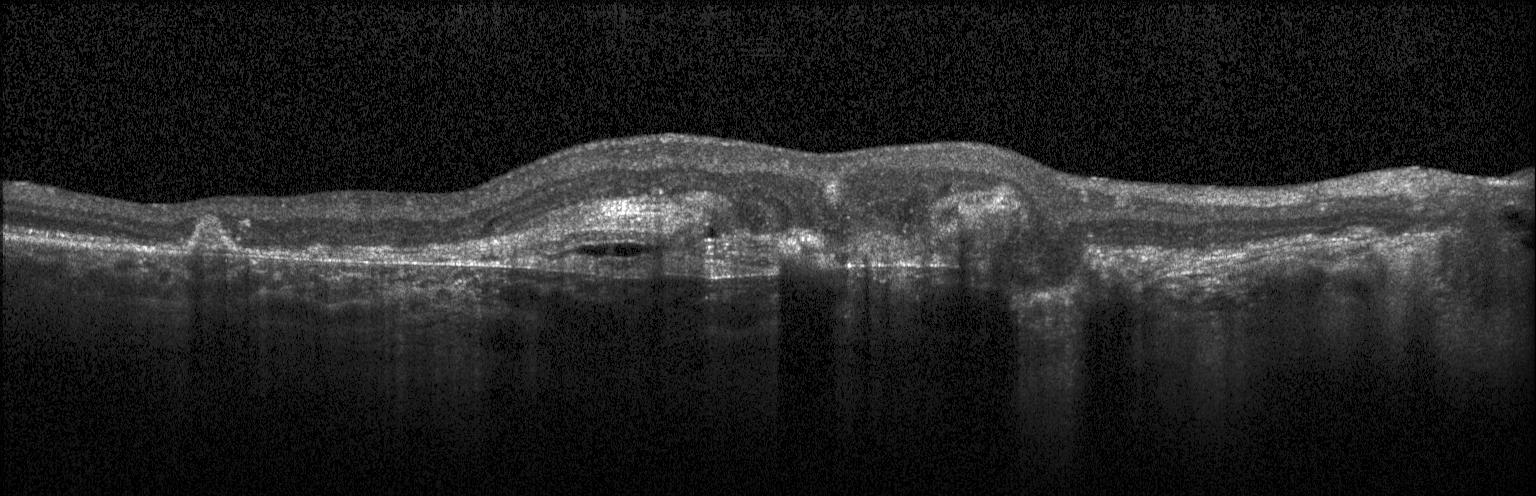

Horizontal scan through the fovea, Heidelberg Spectralis, retinal OCT cross-section. Finding: choroidal neovascularization (CNV).